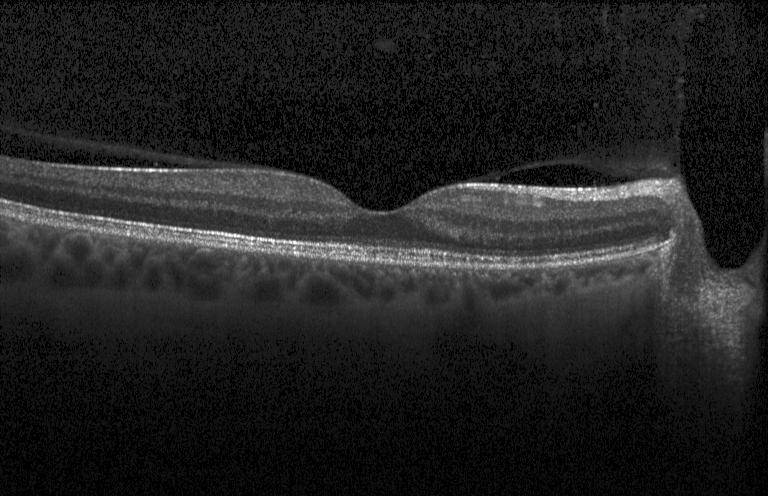 Retinal OCT cross-section; macular scan; Heidelberg Spectralis.
Diagnosis: no CNV, no DME, and no drusen.